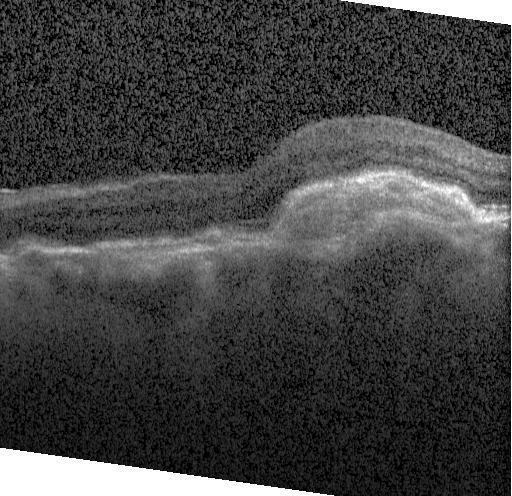

Macular OCT demonstrating a choroidal neovascular membrane.